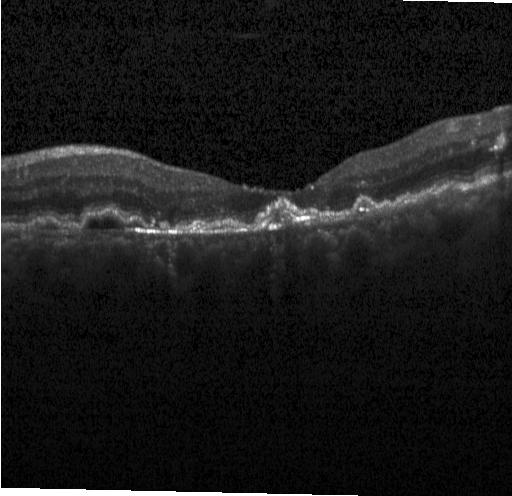 Fovea-centered · acquired on a Heidelberg Spectralis · SD-OCT · optical coherence tomography scan
Diagnosis: choroidal neovascularization.